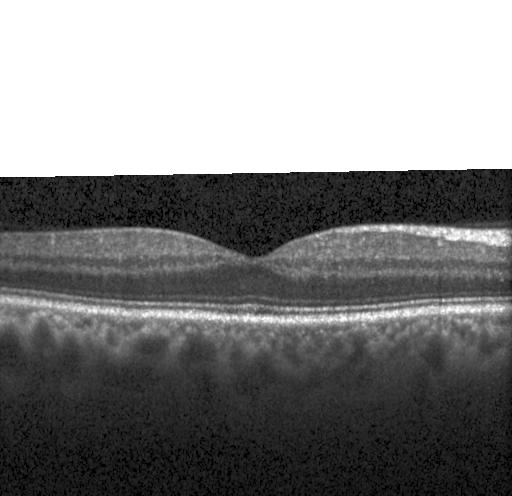
OCT finding: no choroidal neovascularization, no diabetic macular edema, and no drusen.